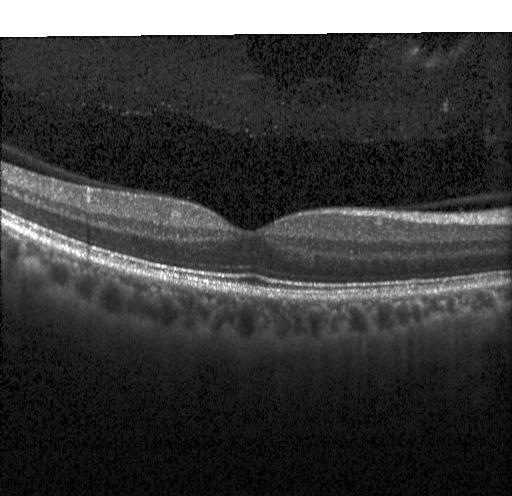 Heidelberg Spectralis OCT system; optical coherence tomography B-scan; through the macula — Assessment: no evidence of CNV, DME, or drusen.